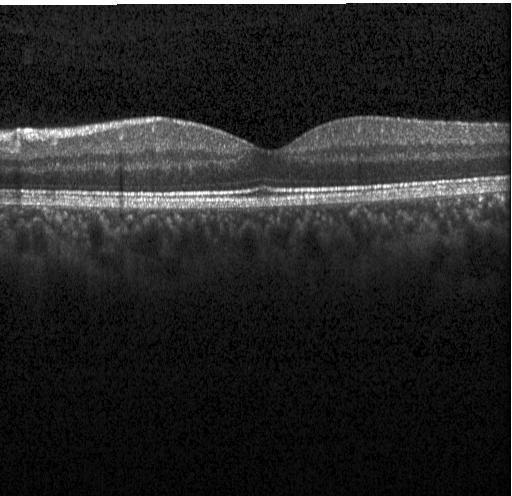

This B-scan demonstrates no choroidal neovascularization, no diabetic macular edema, and no drusen.